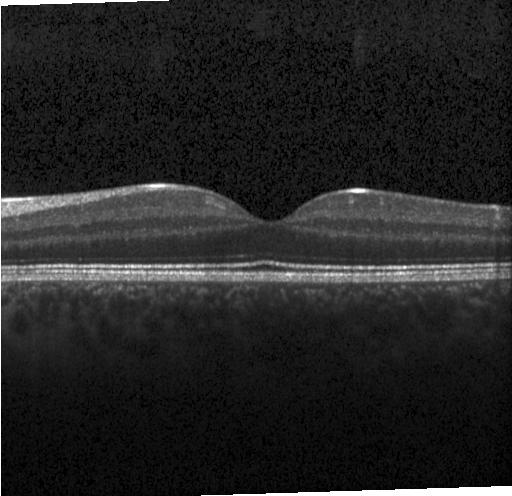 OCT finding: no evidence of choroidal neovascularization, diabetic macular edema, or drusen.